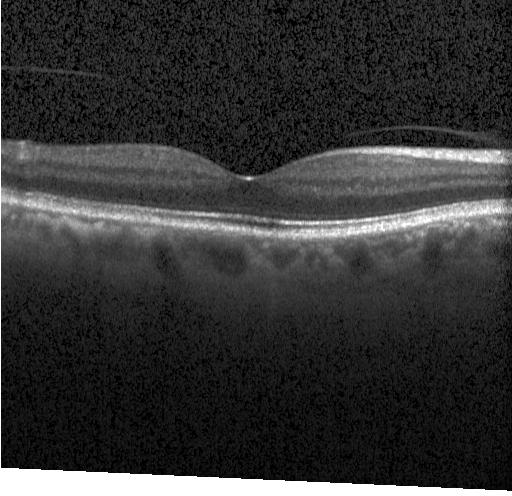
OCT B-scan.
OCT finding: neither choroidal neovascularization, diabetic macular edema, nor drusen.